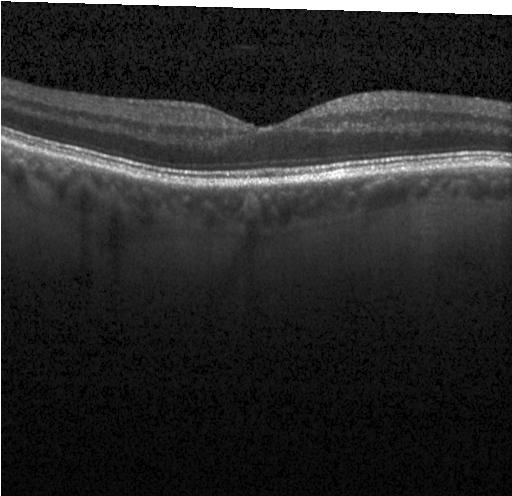
Optical coherence tomography scan; fovea-centered; Heidelberg Spectralis
Diagnosis: neither choroidal neovascularization, diabetic macular edema, nor drusen.